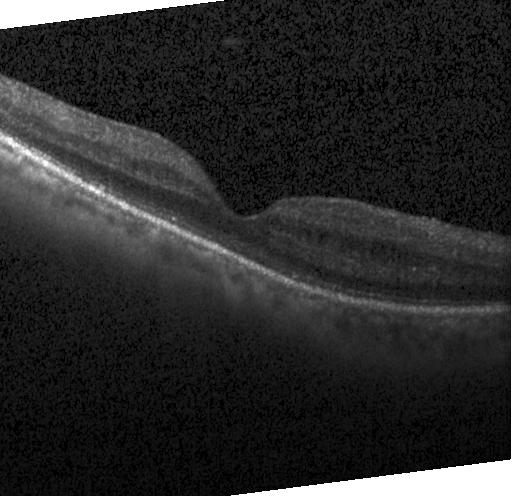 OCT B-scan. This B-scan demonstrates diabetic macular edema.